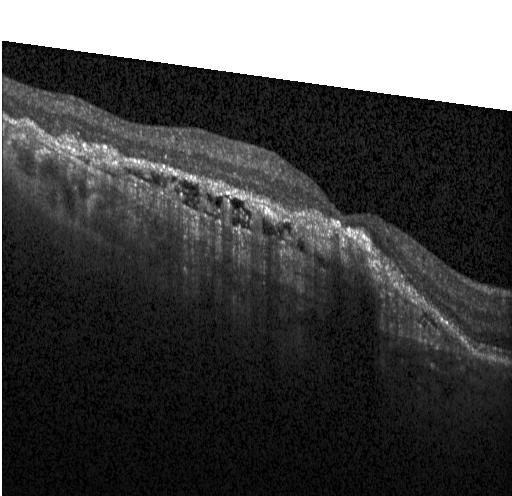 Macular OCT demonstrating a choroidal neovascular membrane.